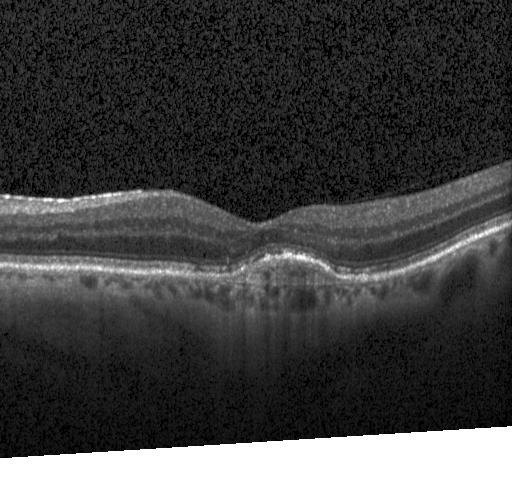 Fovea-centered. Retinal OCT B-scan. Heidelberg Spectralis.
Diagnosis: a choroidal neovascular membrane.